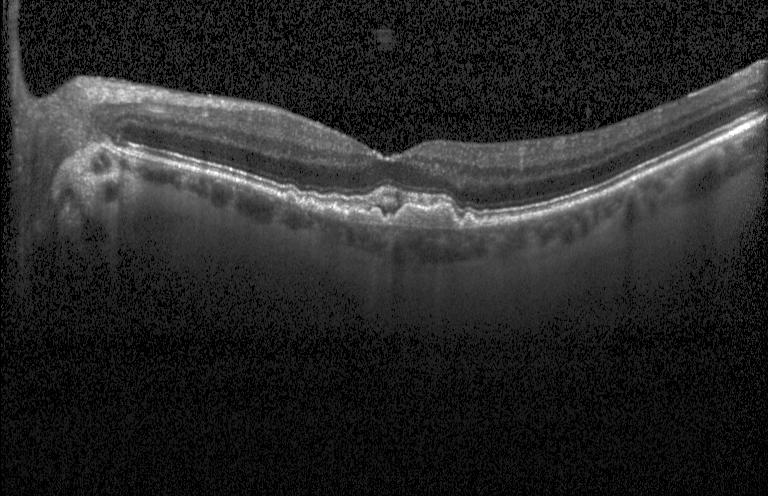
Finding: sub-RPE drusenoid deposits.